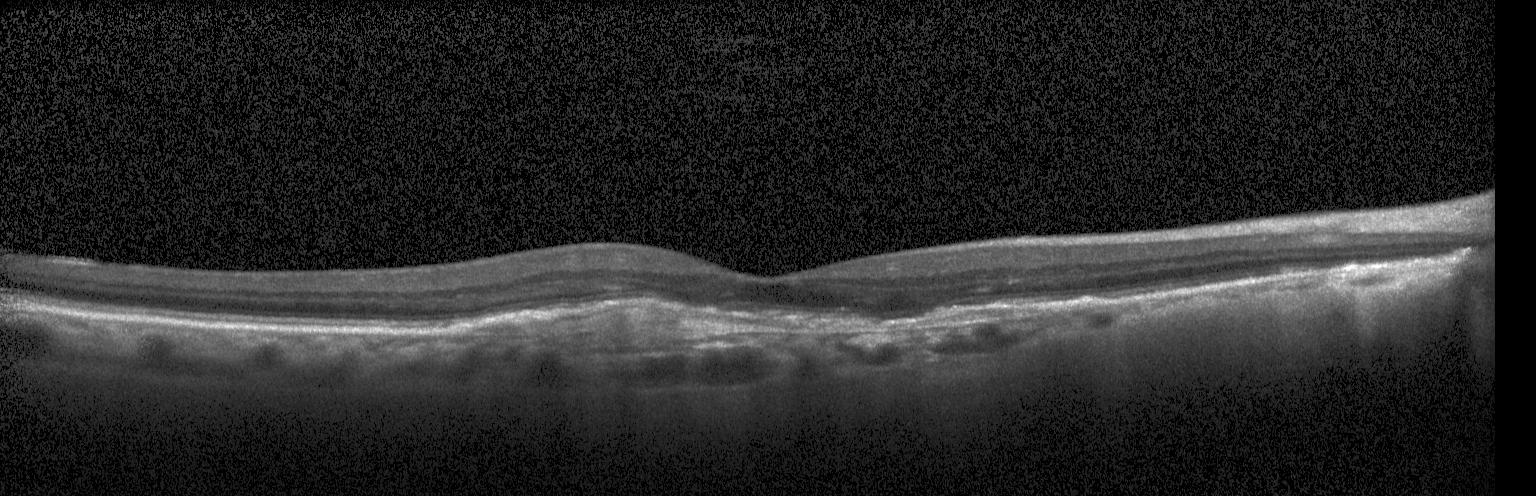 Heidelberg Spectralis OCT system · OCT line scan. Finding: choroidal neovascularization.